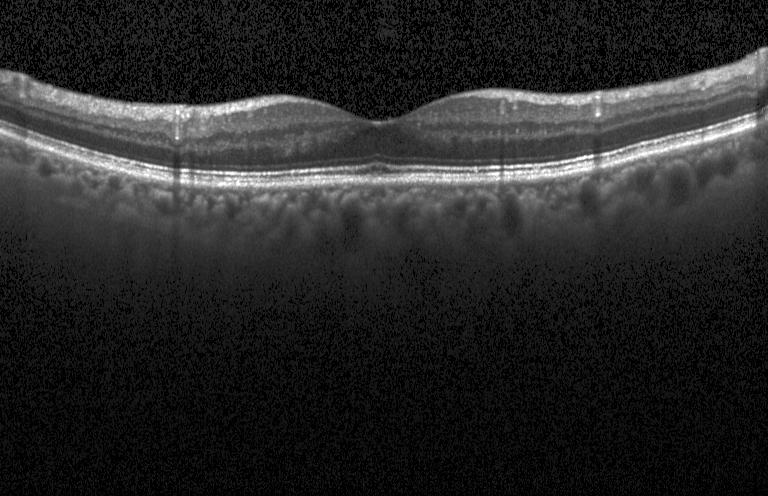

No choroidal neovascularization, no diabetic macular edema, and no drusen.